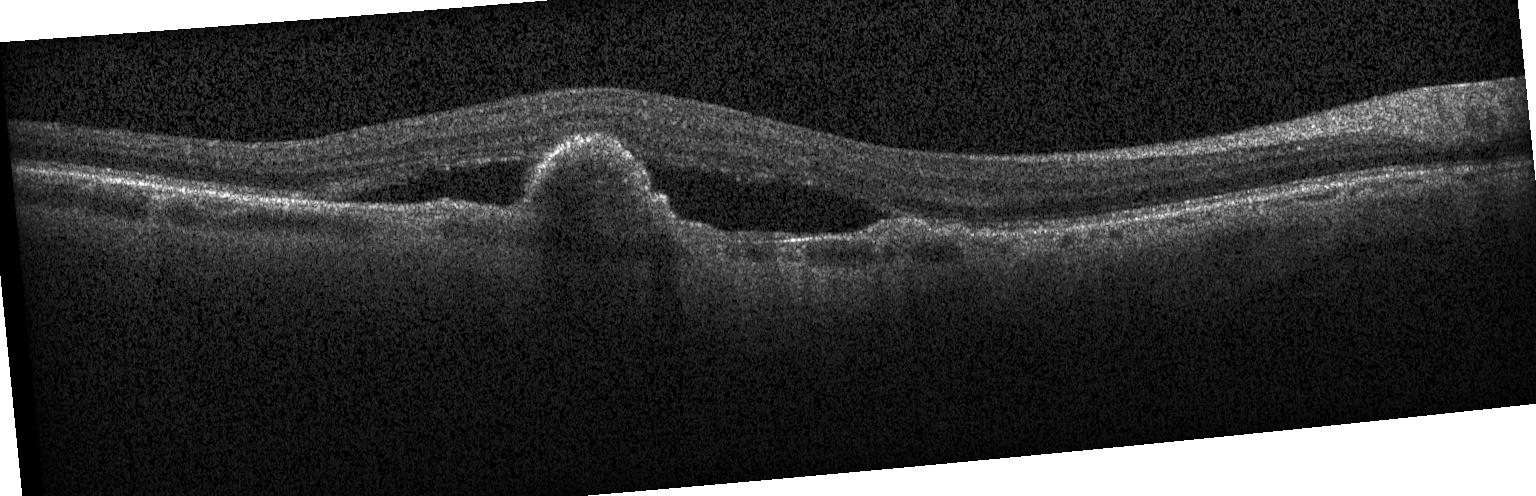

The scan shows CNV.